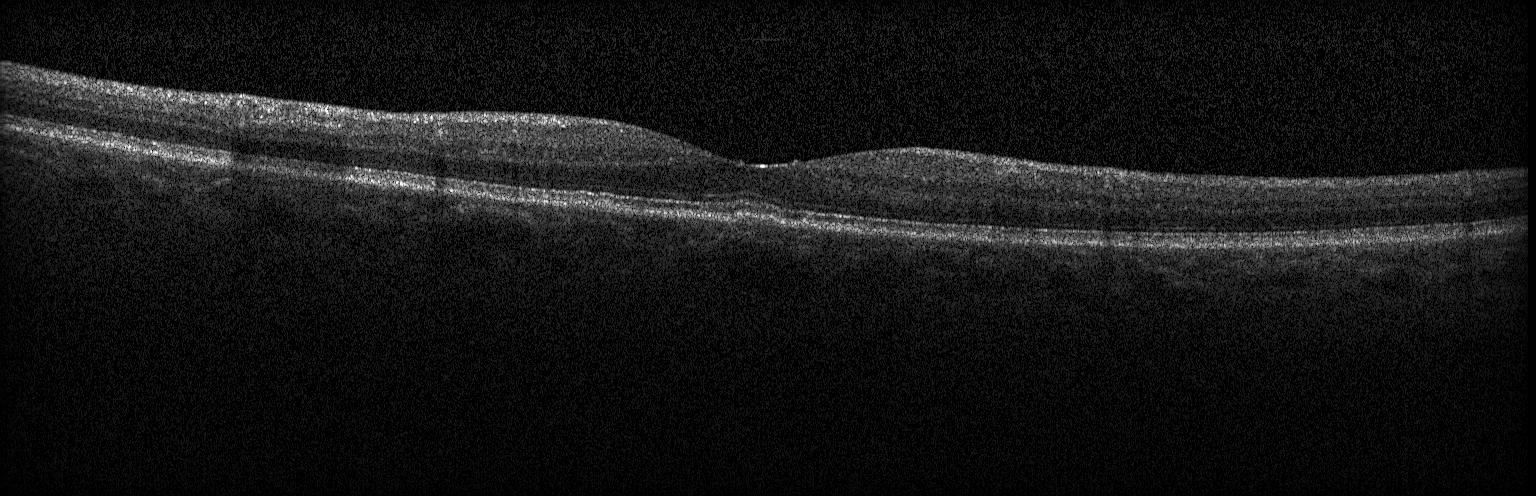

Spectral-domain OCT · instrument: Heidelberg Spectralis · horizontal scan through the fovea · optical coherence tomography scan — This B-scan demonstrates sub-RPE drusenoid deposits.